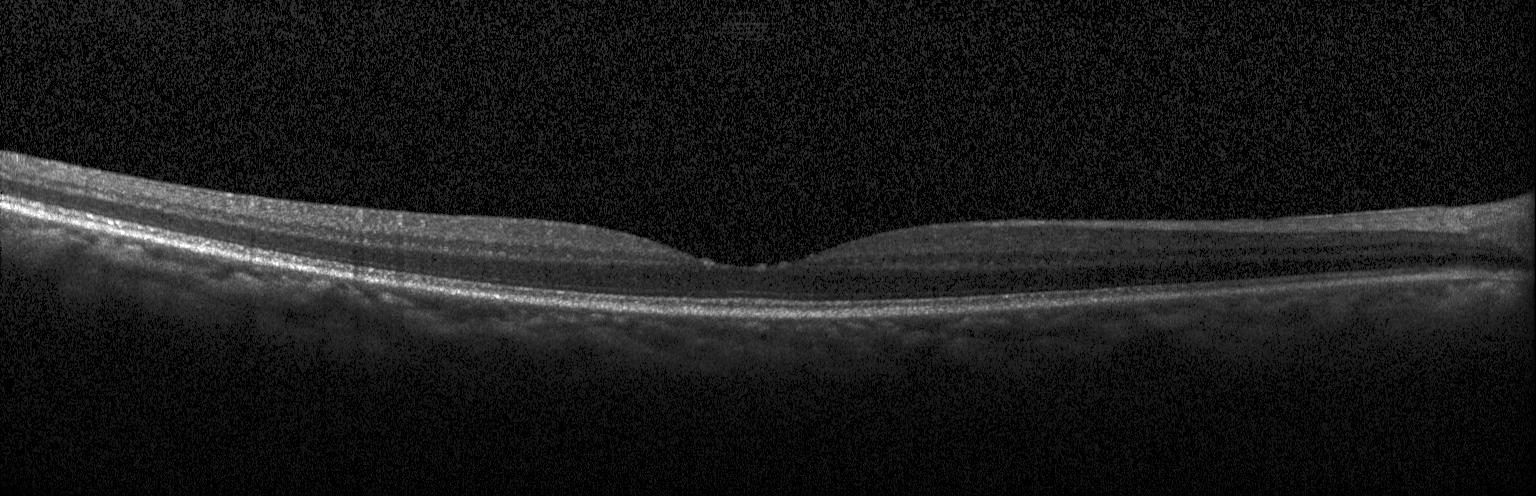
SD-OCT. Macular scan. Optical coherence tomography B-scan.
Finding: no choroidal neovascularization, no diabetic macular edema, and no drusen.